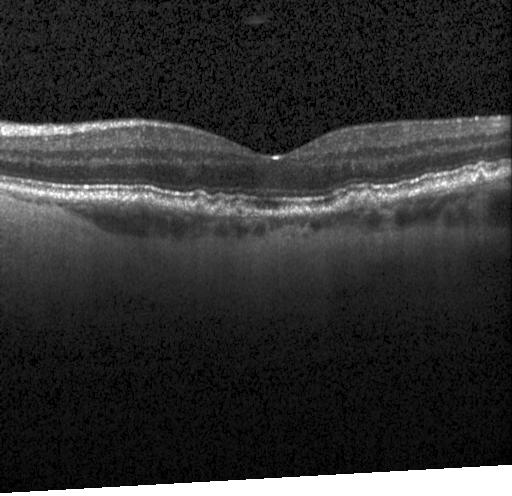 Macular OCT: sub-RPE drusenoid deposits.